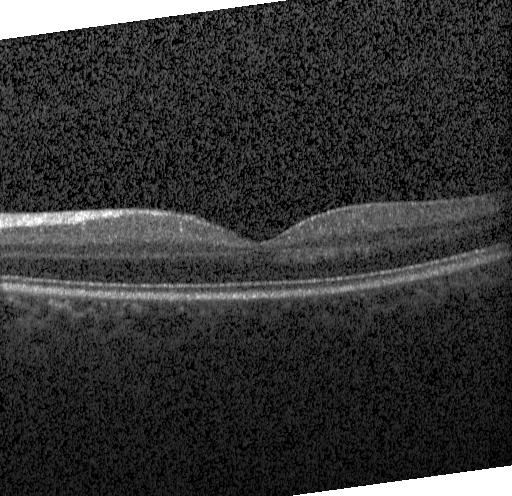 OCT finding: no evidence of CNV, DME, or drusen.